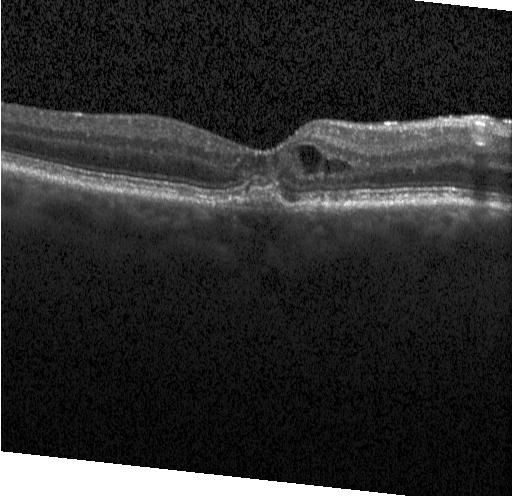

Macular scan · optical coherence tomography scan · spectral-domain OCT.
Diagnosis: choroidal neovascularization (CNV).